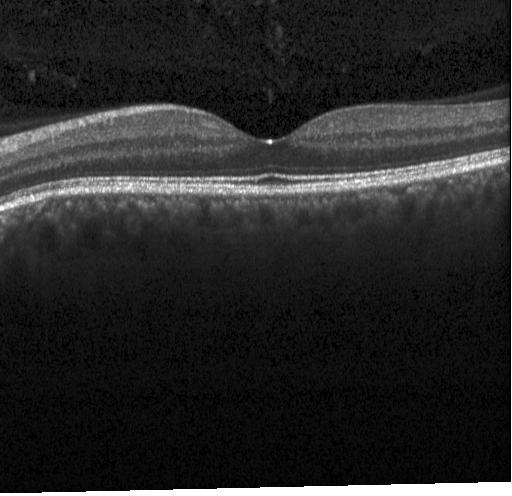
Retinal OCT cross-section showing neither choroidal neovascularization, diabetic macular edema, nor drusen.